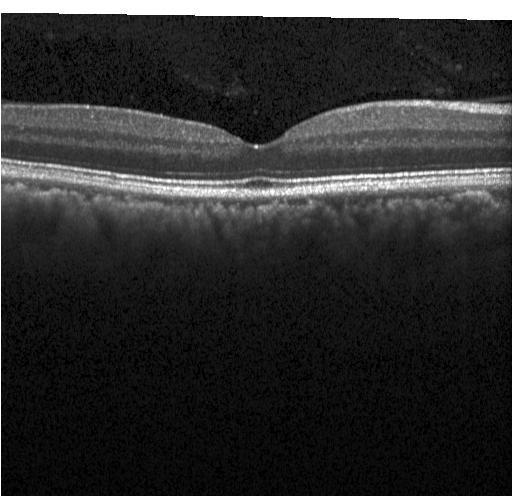 Through the macula · retinal OCT cross-section. Diagnosis: neither CNV, DME, nor drusen.